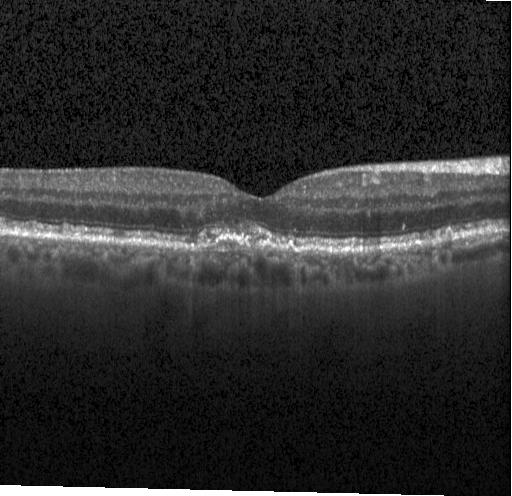

OCT line scan
Finding: a choroidal neovascular membrane.